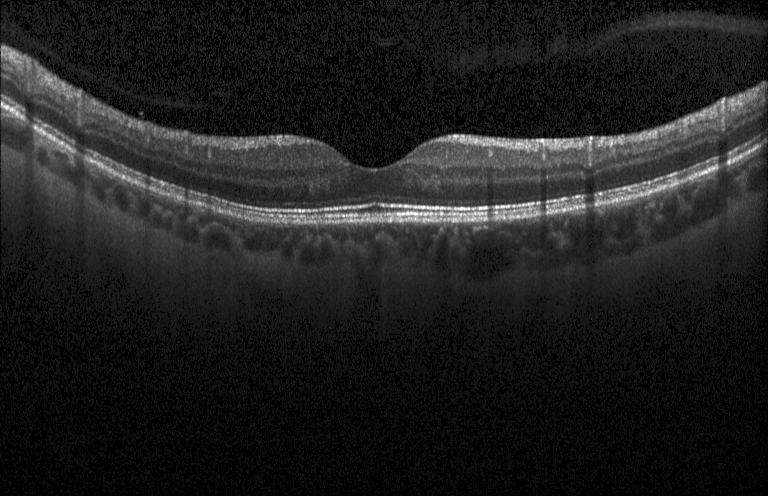
OCT B-scan. Dx: no choroidal neovascularization, diabetic macular edema, or drusen.